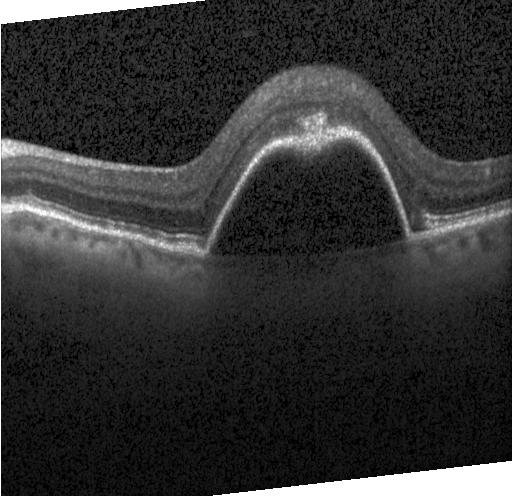 Heidelberg Spectralis; OCT B-scan; spectral-domain OCT — The scan shows CNV.